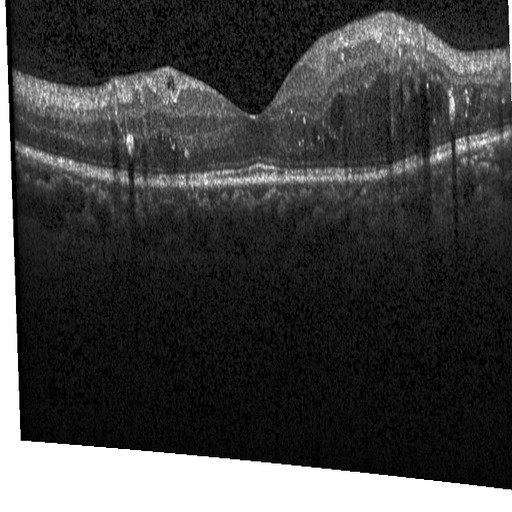 Horizontal scan through the fovea. Spectral-domain optical coherence tomography. Retinal OCT B-scan.
Macular OCT: diabetic macular edema (DME).